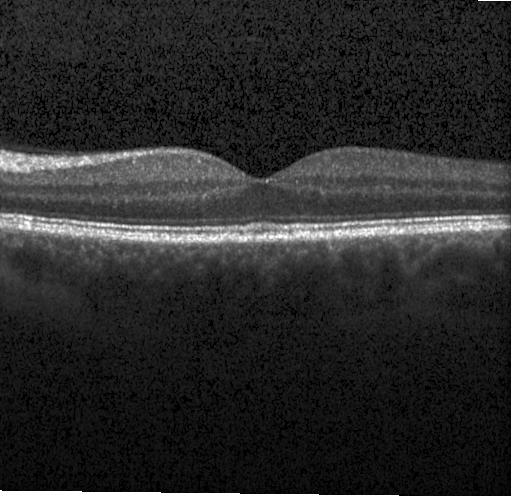

Heidelberg Spectralis; optical coherence tomography B-scan
Impression: no evidence of CNV, DME, or drusen.